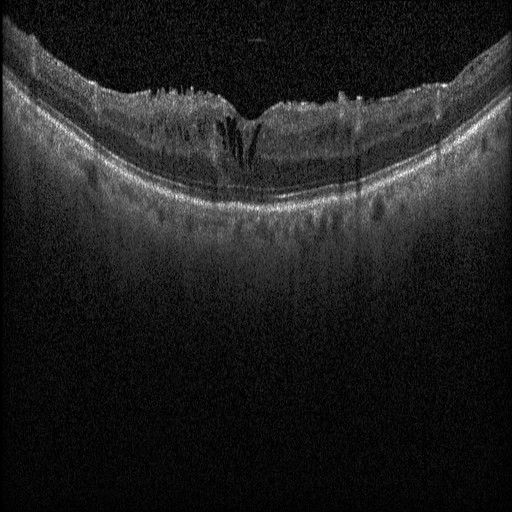
OCT B-scan. Acquired on a Heidelberg Spectralis. Spectral-domain optical coherence tomography. Horizontal scan through the fovea.
Finding: diabetic macular edema.